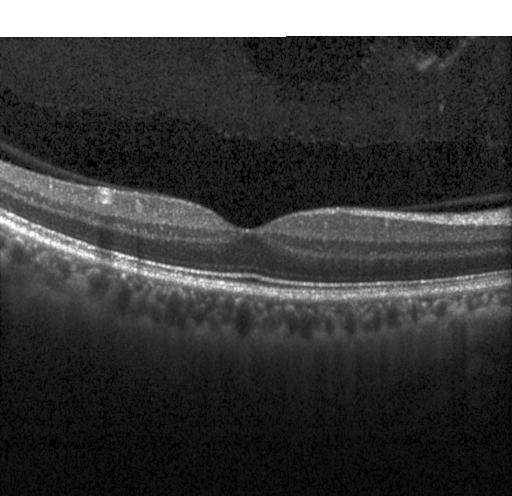

Through the macula. Instrument: Heidelberg Spectralis. Optical coherence tomography scan — Dx: no choroidal neovascularization, no diabetic macular edema, and no drusen.